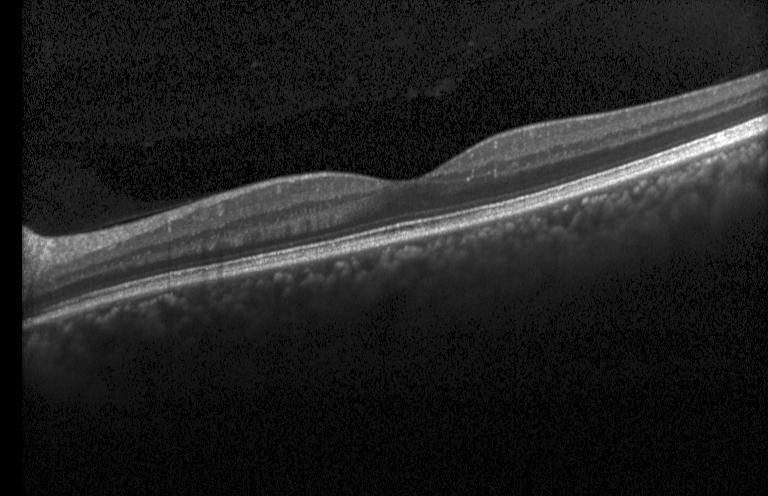

OCT B-scan, Heidelberg Spectralis — Dx: neither choroidal neovascularization, diabetic macular edema, nor drusen.